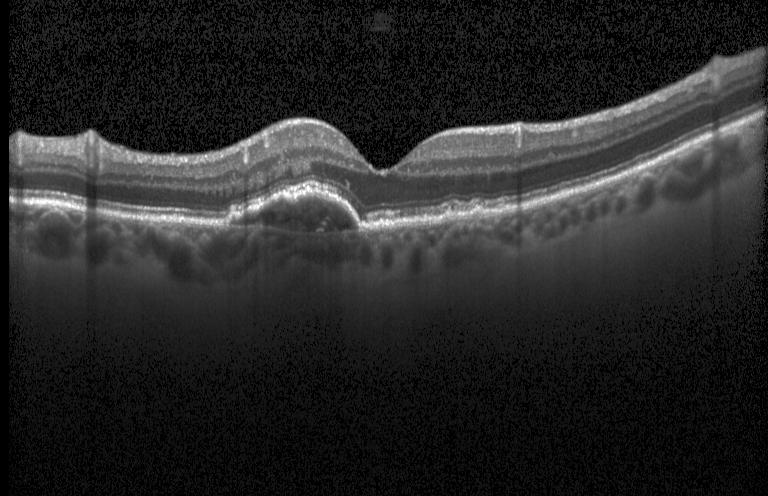 Fovea-centered; retinal OCT B-scan; spectral-domain optical coherence tomography; Heidelberg Spectralis.
Assessment: a choroidal neovascular membrane.